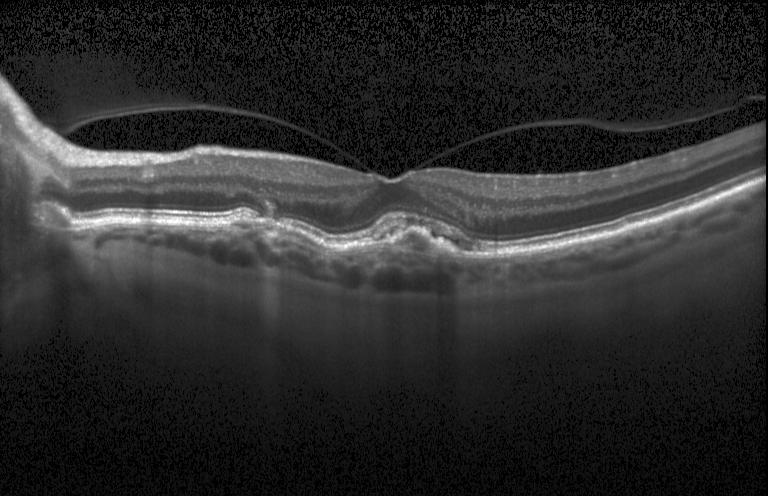
Diagnosis: CNV.